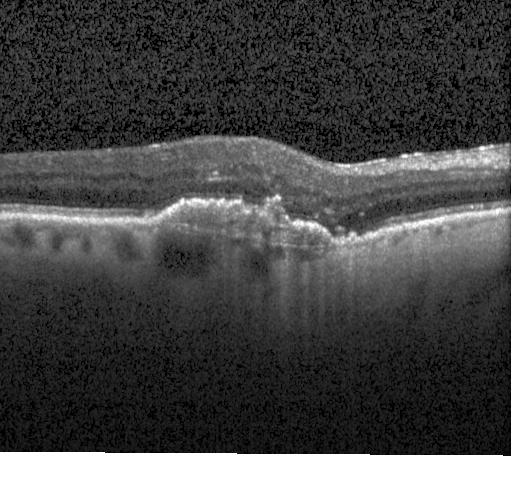 OCT scan showing a choroidal neovascular membrane.